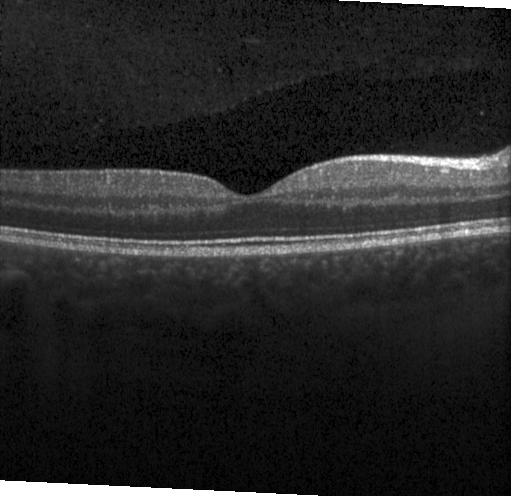
Impression: no evidence of choroidal neovascularization, diabetic macular edema, or drusen.